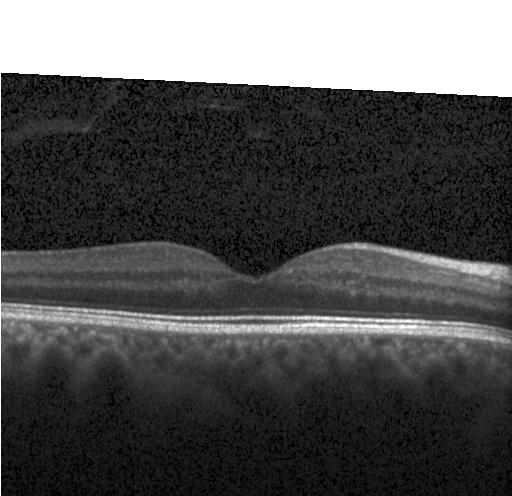 Optical coherence tomography scan — Dx: no choroidal neovascularization, no diabetic macular edema, and no drusen.